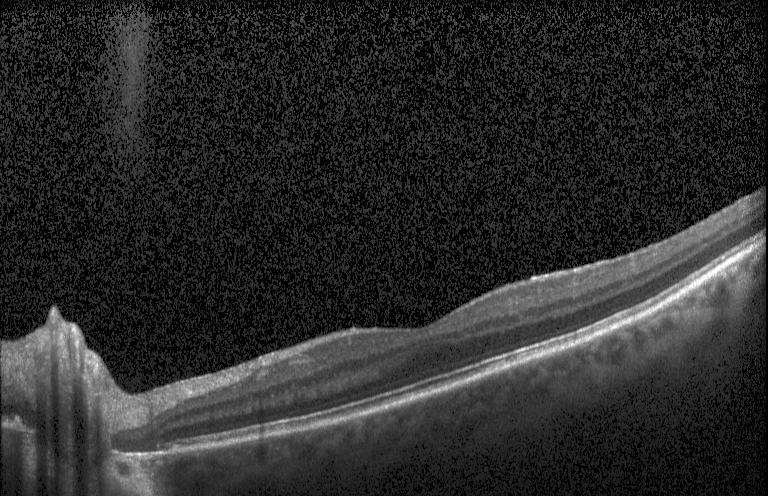

No choroidal neovascularization, no diabetic macular edema, and no drusen.